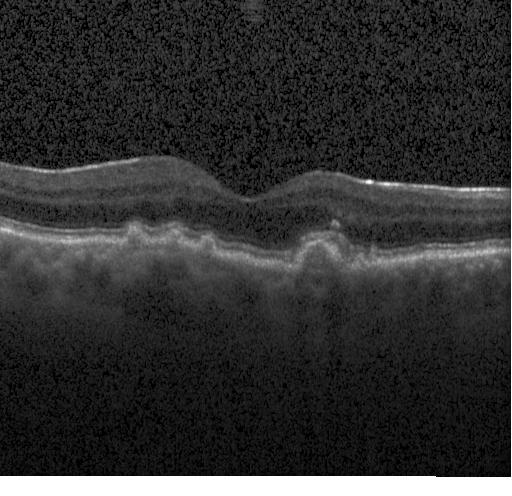 Horizontal scan through the fovea. OCT line scan.
Assessment: sub-RPE drusenoid deposits.